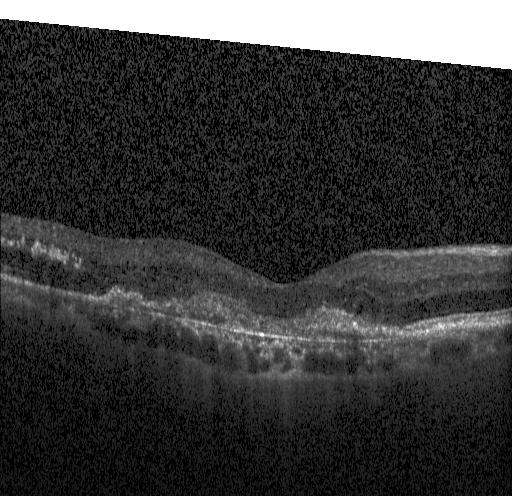

This B-scan demonstrates a choroidal neovascular membrane.